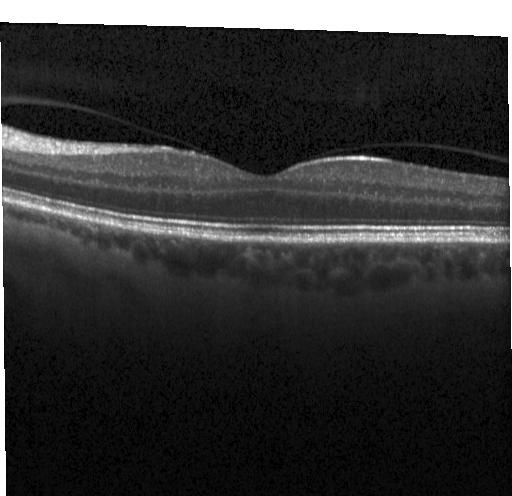

Heidelberg Spectralis · OCT B-scan. Finding: no evidence of choroidal neovascularization, diabetic macular edema, or drusen.